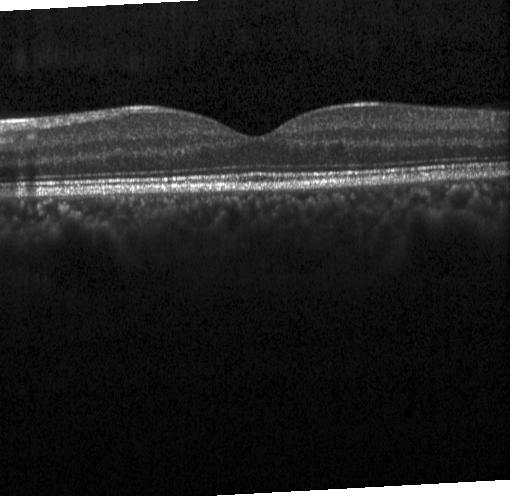 Macular OCT demonstrating no choroidal neovascularization, diabetic macular edema, or drusen.